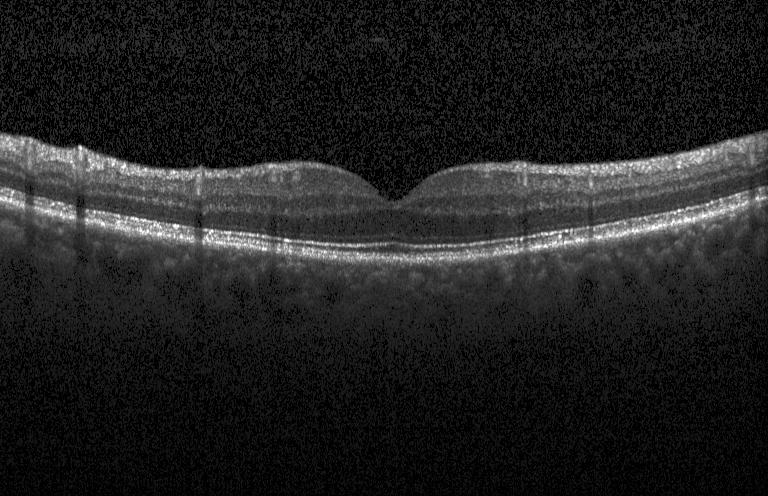 OCT line scan · Heidelberg Spectralis OCT system · SD-OCT. Finding: neither choroidal neovascularization, diabetic macular edema, nor drusen.